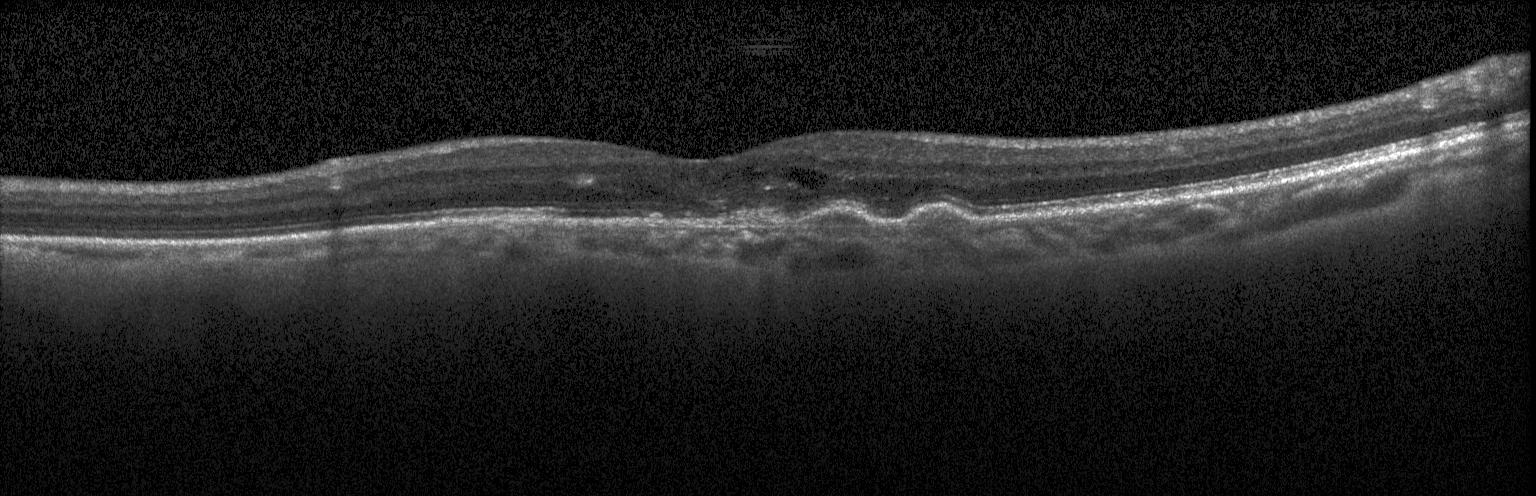
Through the macula. Acquired on a Heidelberg Spectralis. Retinal OCT cross-section. Spectral-domain OCT — Impression: CNV.